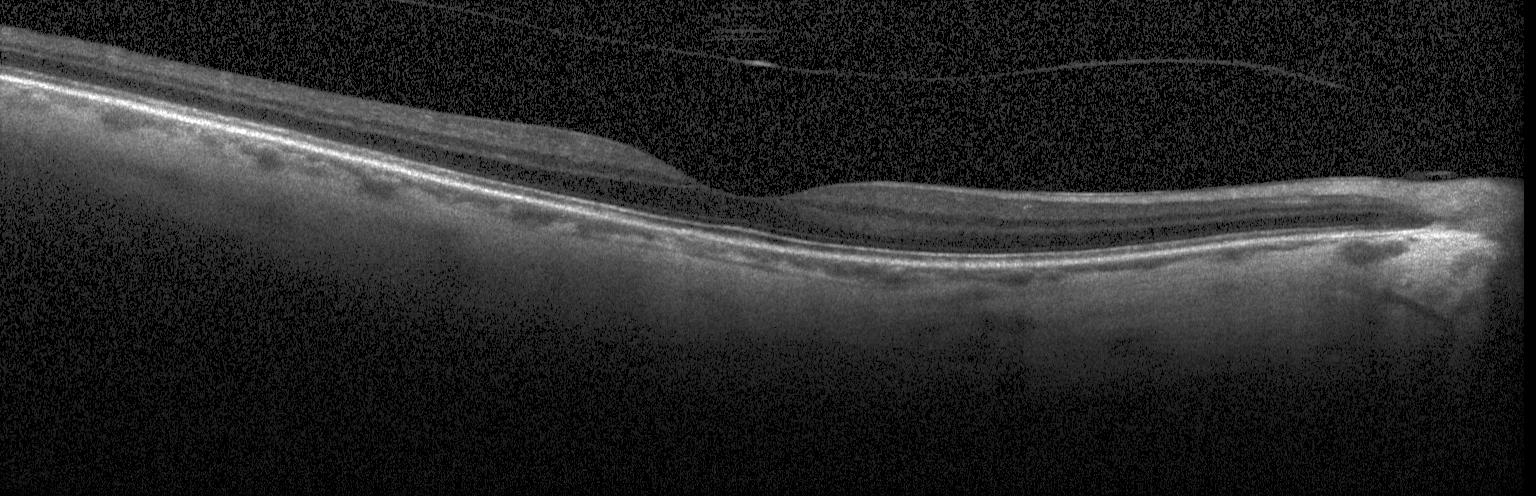

Retinal OCT cross-section
OCT finding: no choroidal neovascularization, diabetic macular edema, or drusen.